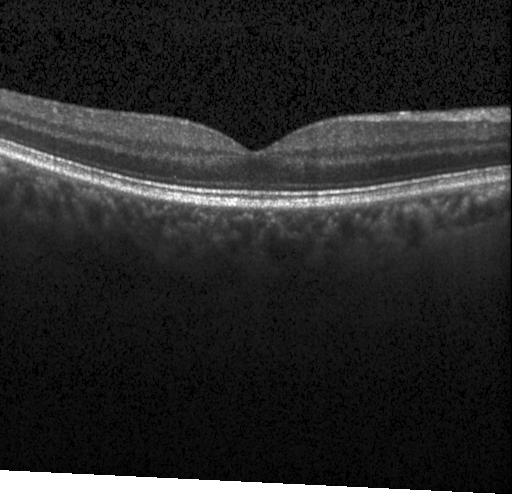 Centered on the fovea · Heidelberg Spectralis OCT system · OCT line scan. Impression: no choroidal neovascularization, diabetic macular edema, or drusen.